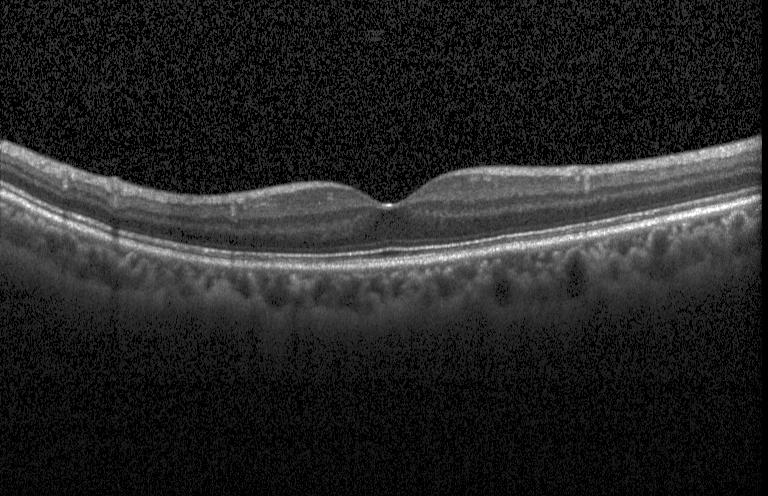 Spectral-domain optical coherence tomography; retinal OCT cross-section; centered on the fovea
No CNV, DME, or drusen.